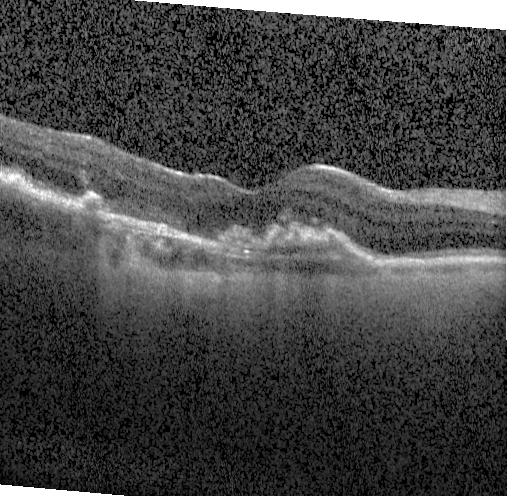 Retinal OCT B-scan. Spectral-domain OCT. Impression: choroidal neovascularization (CNV).